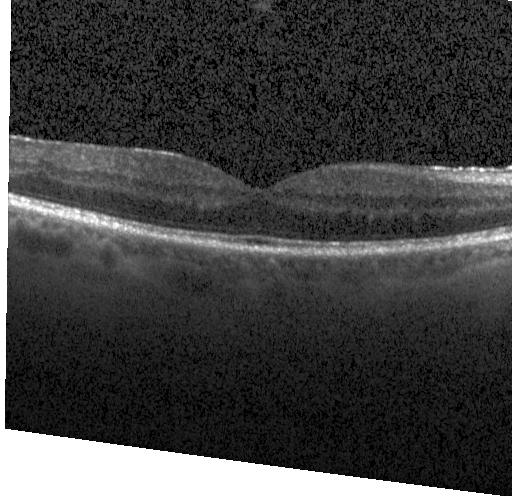
Retinal OCT cross-section showing no evidence of choroidal neovascularization, diabetic macular edema, or drusen.